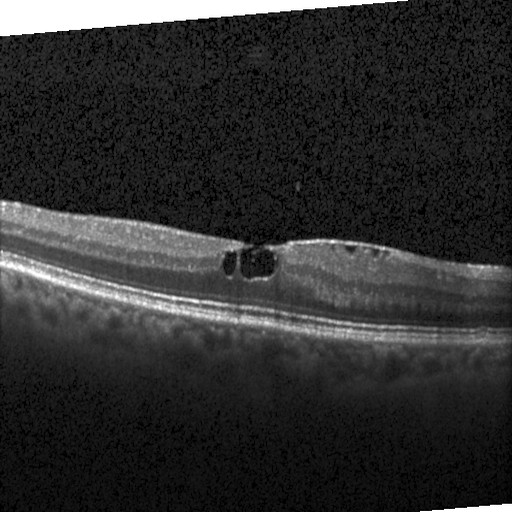
OCT B-scan. Diabetic macular edema.